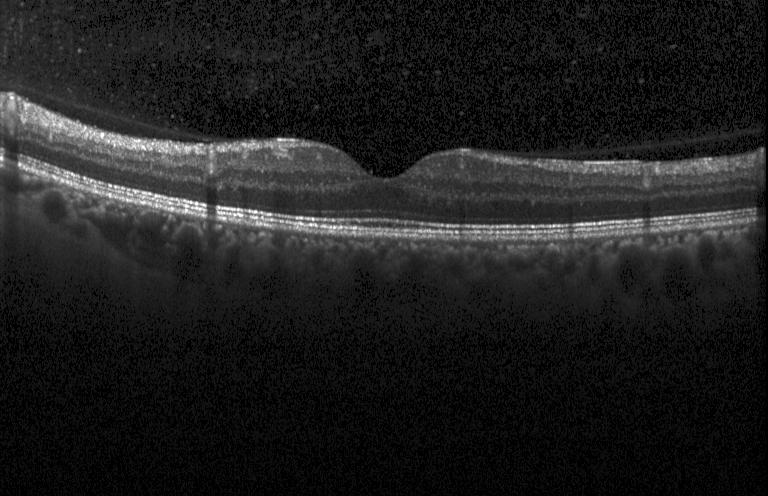 OCT finding: neither choroidal neovascularization, diabetic macular edema, nor drusen.